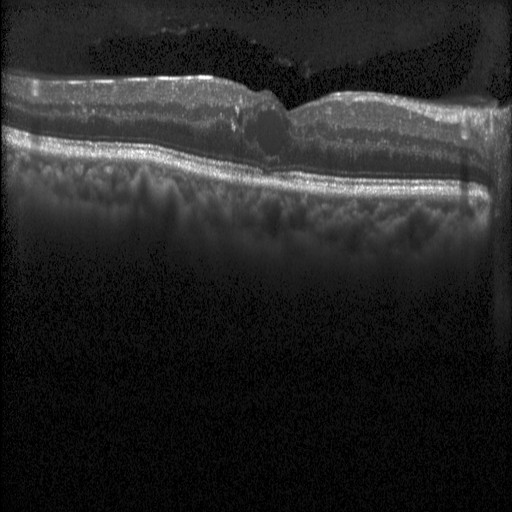
Macular OCT: diabetic macular edema.